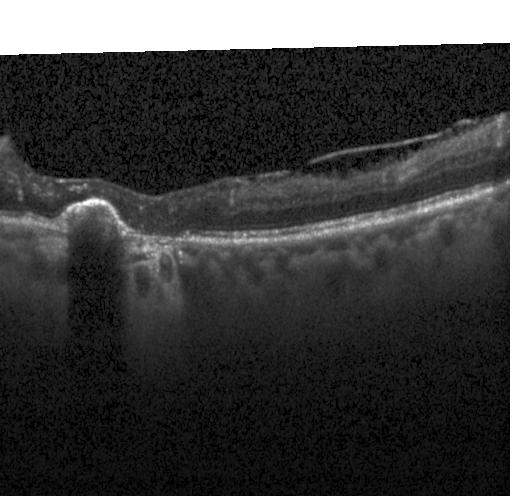

Retinal OCT cross-section; macular scan
OCT finding: a choroidal neovascular membrane.